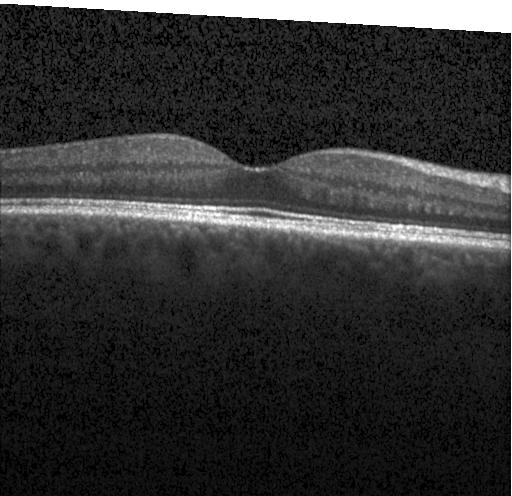 Macular OCT: no evidence of choroidal neovascularization, diabetic macular edema, or drusen.